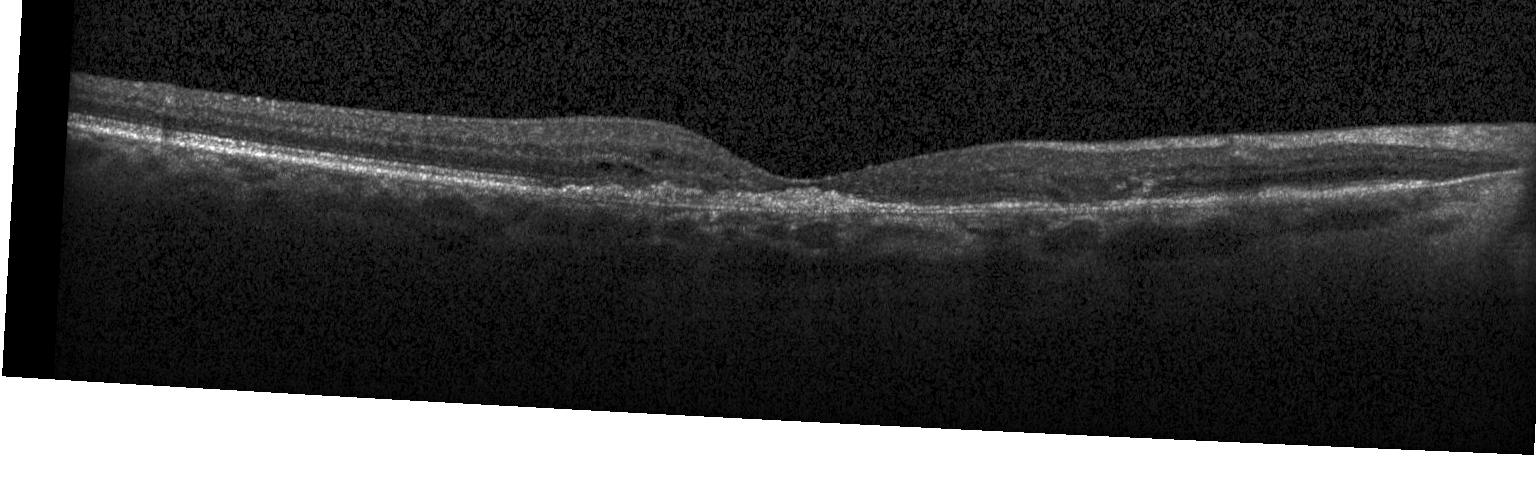 Finding: a choroidal neovascular membrane.